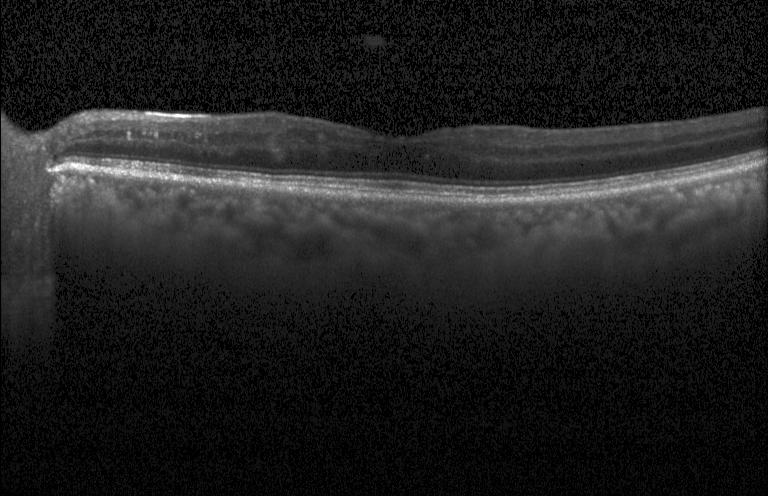
Centered on the fovea, spectral-domain OCT, OCT B-scan — Dx: no evidence of choroidal neovascularization, diabetic macular edema, or drusen.